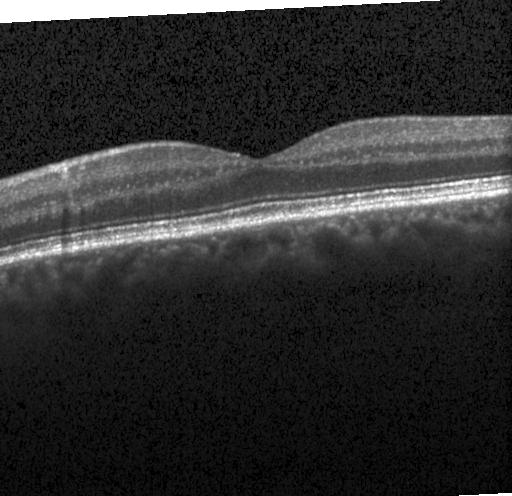
Macular OCT demonstrating no CNV, DME, or drusen.